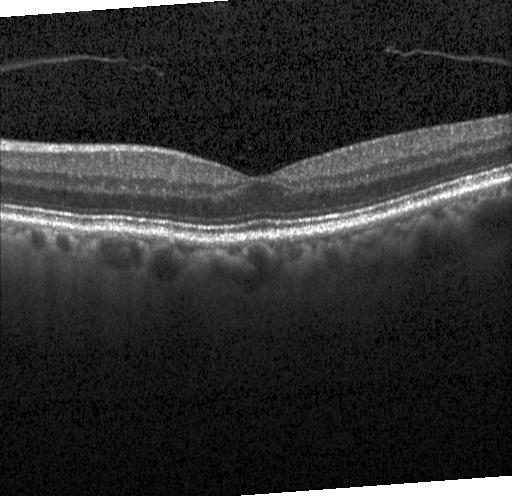
Macular OCT: neither choroidal neovascularization, diabetic macular edema, nor drusen.